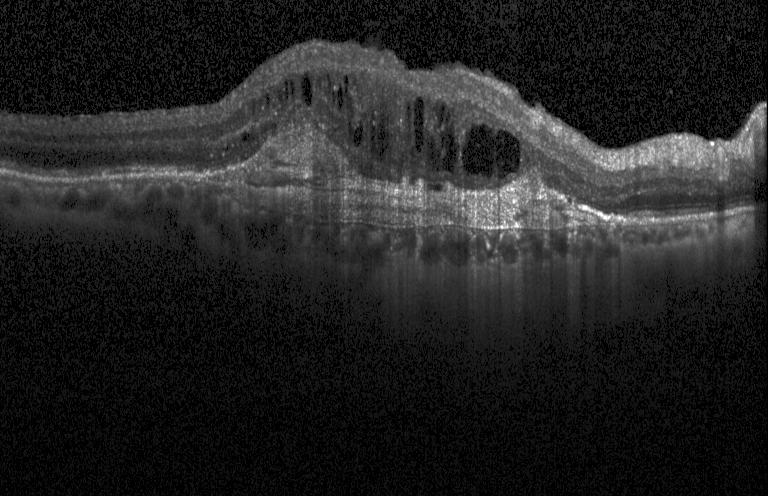
This B-scan demonstrates choroidal neovascularization (CNV).